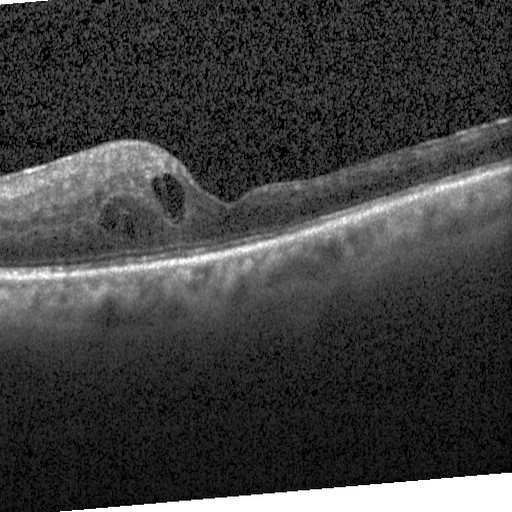 Impression: diabetic macular edema (DME).